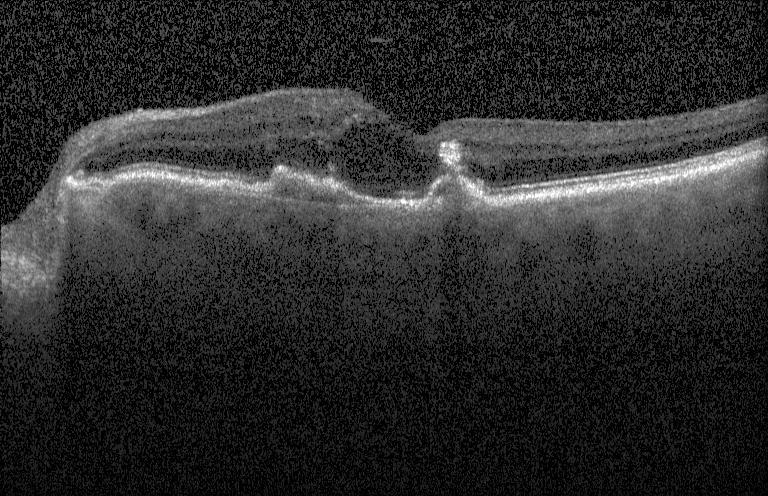

Assessment: a choroidal neovascular membrane.